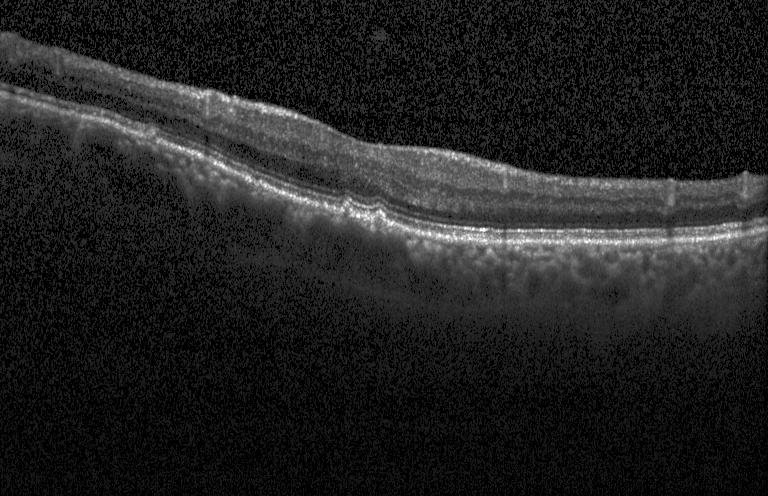 Retinal OCT B-scan. Finding: sub-RPE drusenoid deposits.